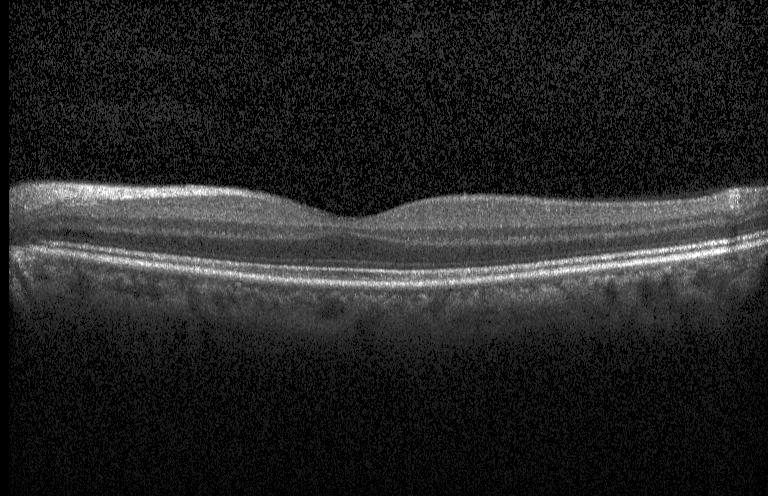 Diagnosis: no evidence of choroidal neovascularization, diabetic macular edema, or drusen.